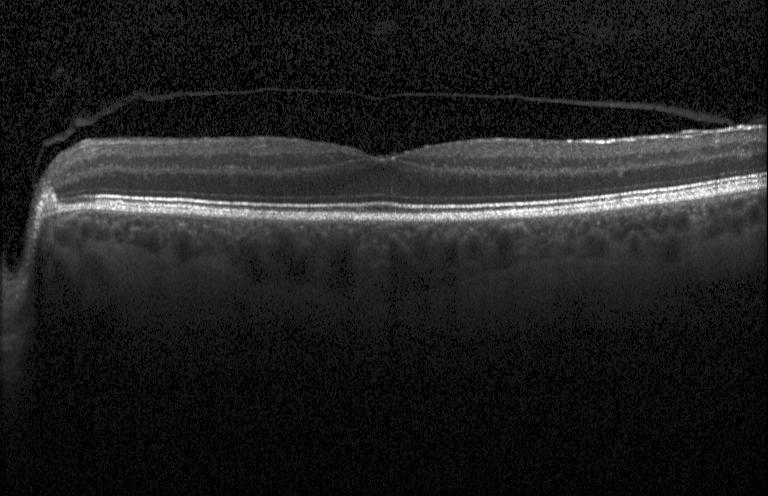

Optical coherence tomography B-scan; horizontal scan through the fovea; Heidelberg Spectralis OCT system
Finding: no evidence of CNV, DME, or drusen.